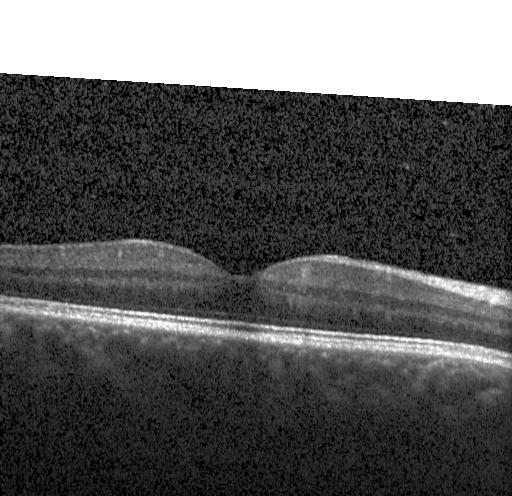 Optical coherence tomography scan · acquired on a Heidelberg Spectralis — Diagnosis: no evidence of choroidal neovascularization, diabetic macular edema, or drusen.